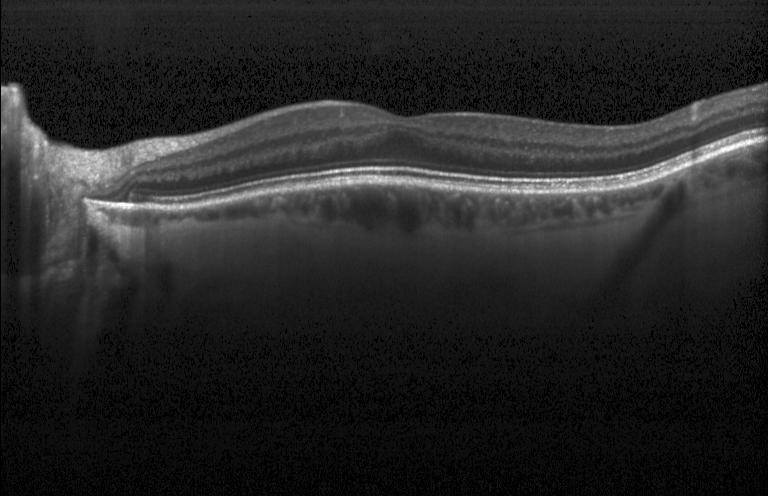
Spectral-domain OCT B-scan: neither CNV, DME, nor drusen.